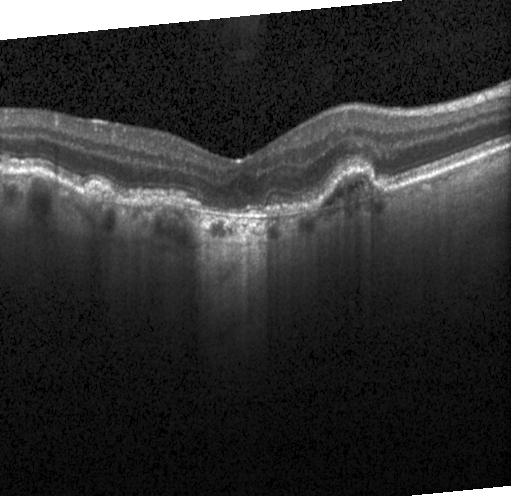 Heidelberg Spectralis OCT system, OCT B-scan, spectral-domain optical coherence tomography.
OCT finding: choroidal neovascularization (CNV).